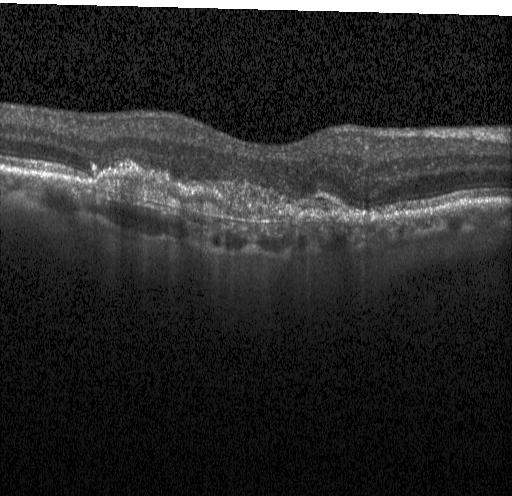
Instrument: Heidelberg Spectralis; through the macula; OCT B-scan. Diagnosis: a choroidal neovascular membrane.